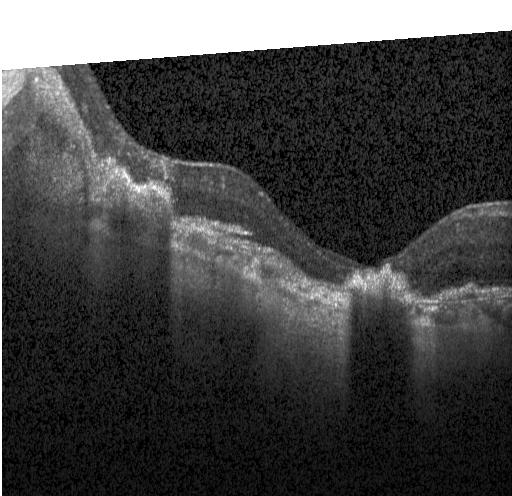 Impression: a choroidal neovascular membrane.